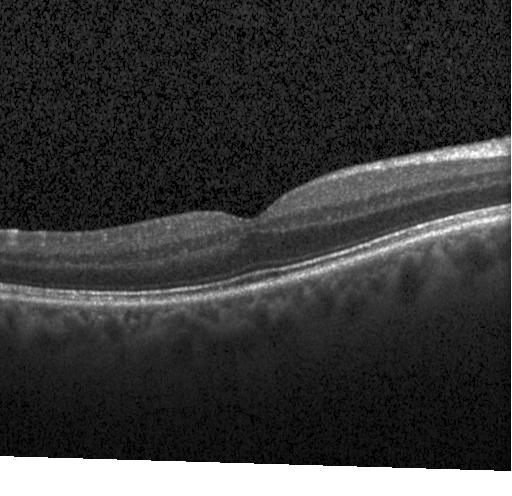
SD-OCT; OCT B-scan. Impression: neither CNV, DME, nor drusen.